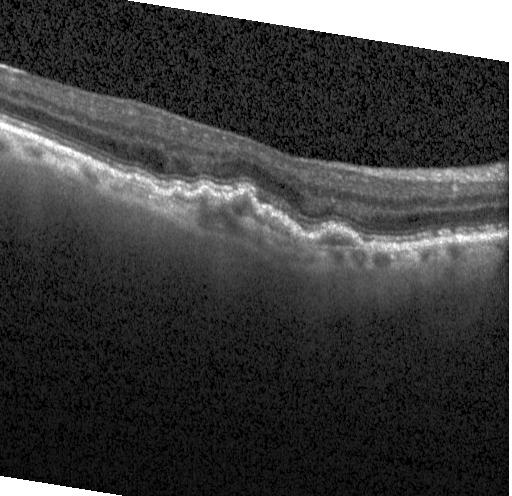

Retinal OCT B-scan; spectral-domain optical coherence tomography; instrument: Heidelberg Spectralis. Macular OCT: choroidal neovascularization.